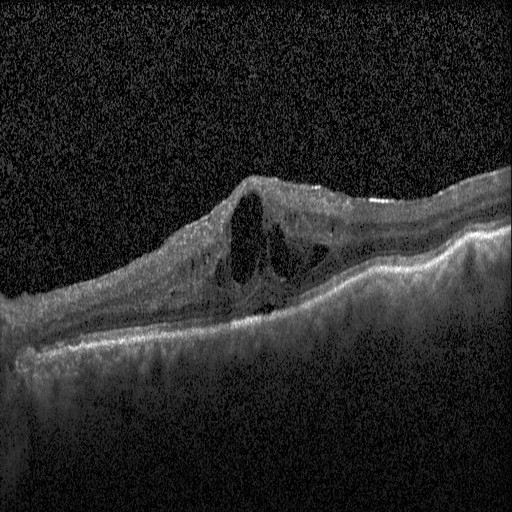
OCT finding: diabetic macular edema (DME).